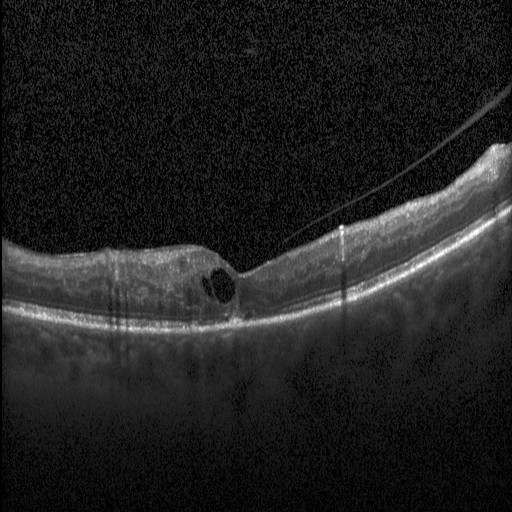
OCT scan showing diabetic macular edema (DME).